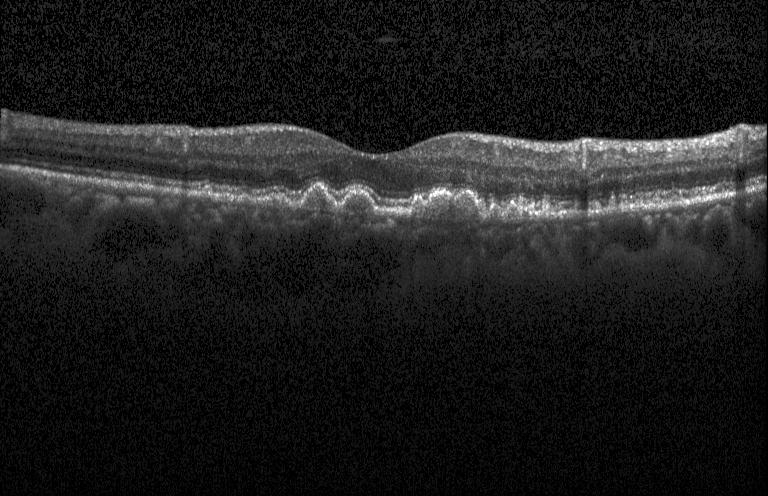 Retinal OCT B-scan. Macular scan. Spectral-domain OCT. Acquired on a Heidelberg Spectralis. Drusen.